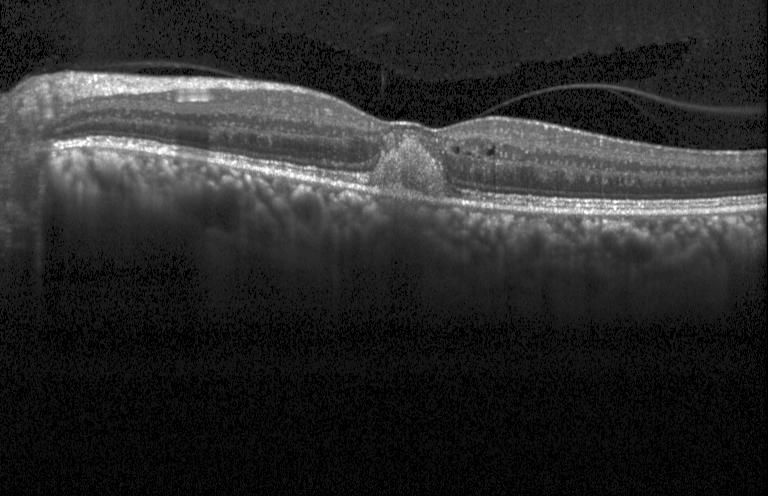
Retinal OCT cross-section — This B-scan demonstrates CNV.